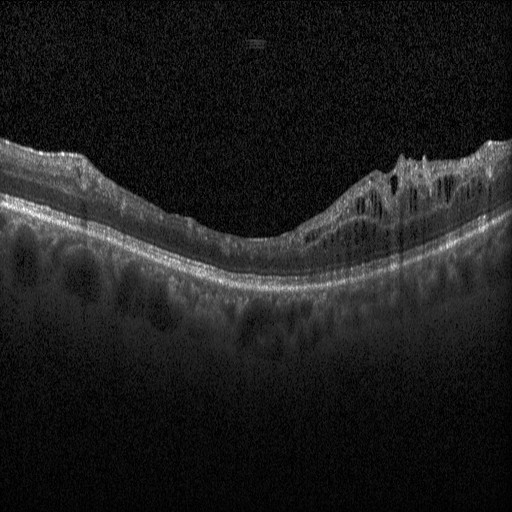
OCT finding: DME.